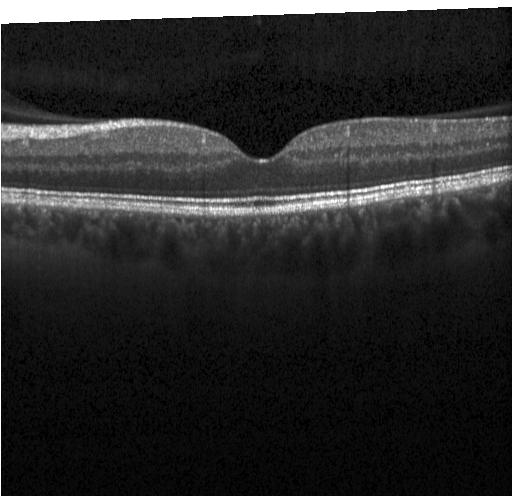 OCT scan showing neither CNV, DME, nor drusen.